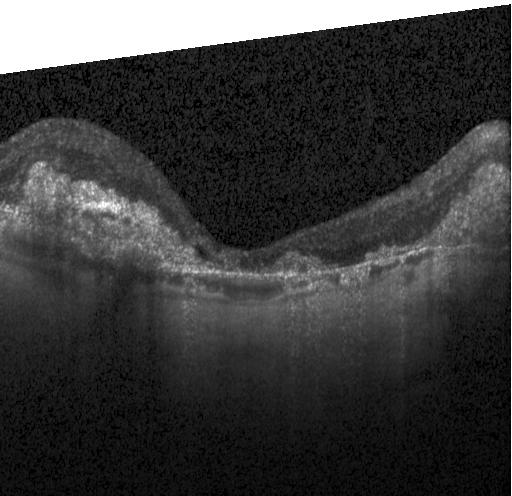
Retinal OCT cross-section, centered on the fovea — Finding: choroidal neovascularization.